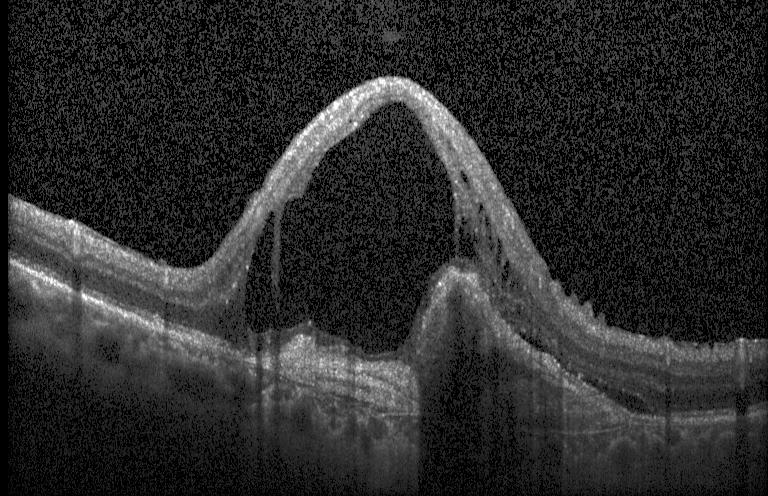
Spectral-domain OCT; Heidelberg Spectralis OCT system; horizontal scan through the fovea; retinal OCT B-scan.
This B-scan demonstrates a choroidal neovascular membrane.